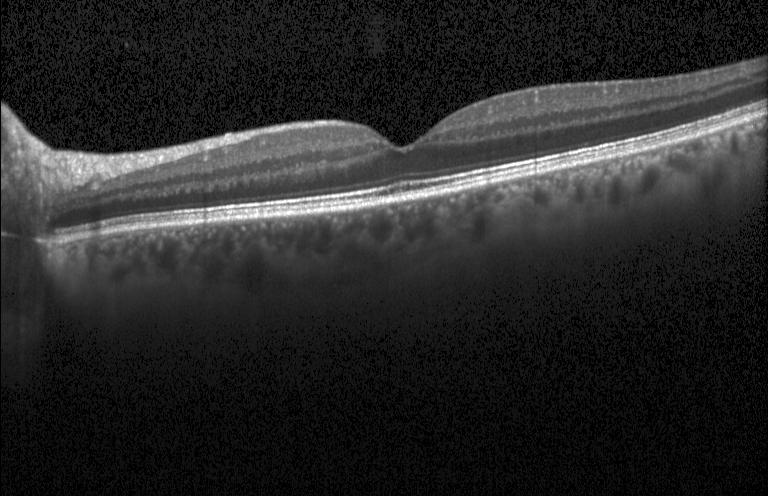 Impression: neither choroidal neovascularization, diabetic macular edema, nor drusen.